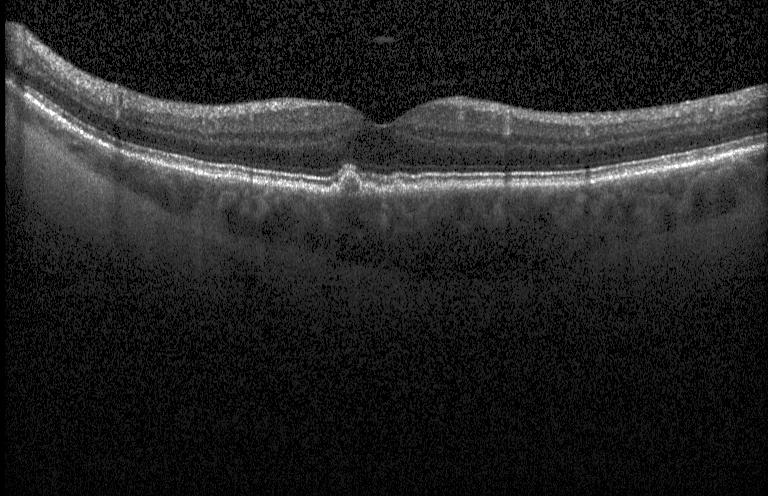

Retinal OCT B-scan
Impression: drusen.